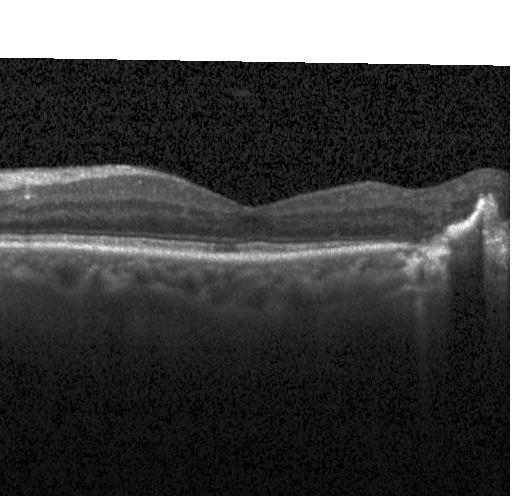
Optical coherence tomography scan, SD-OCT, centered on the fovea, acquired on a Heidelberg Spectralis
Diagnosis: a choroidal neovascular membrane.